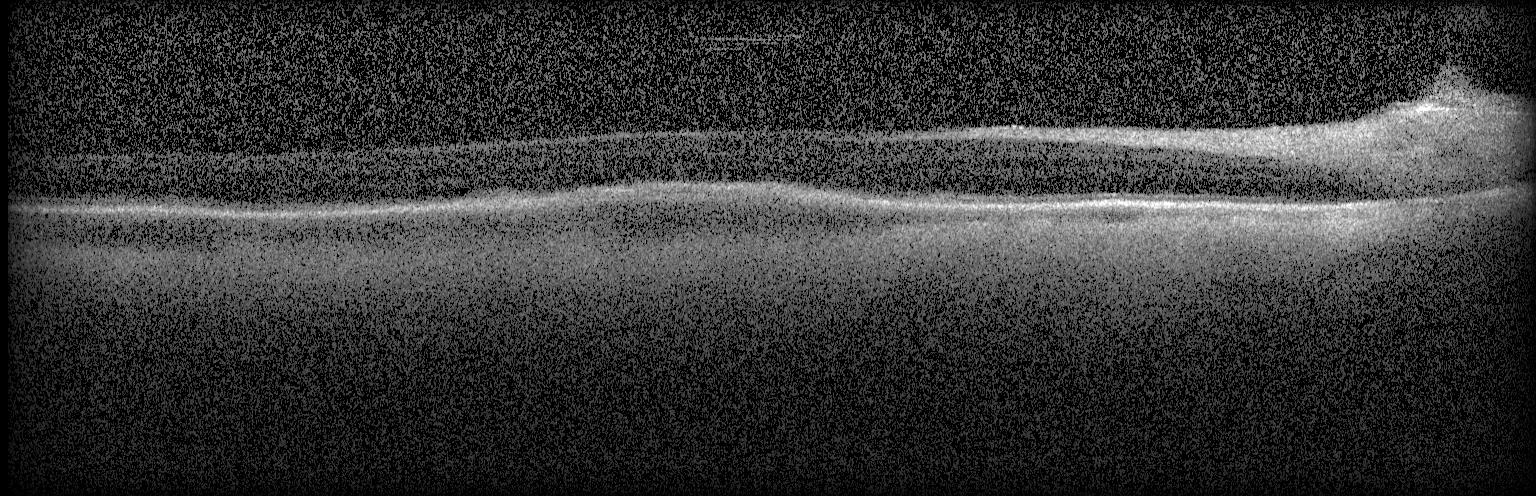
Retinal OCT cross-section.
Assessment: a choroidal neovascular membrane.